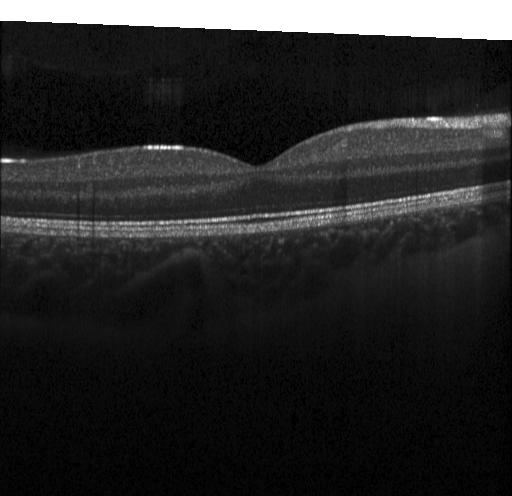 Macular OCT demonstrating no choroidal neovascularization, no diabetic macular edema, and no drusen.